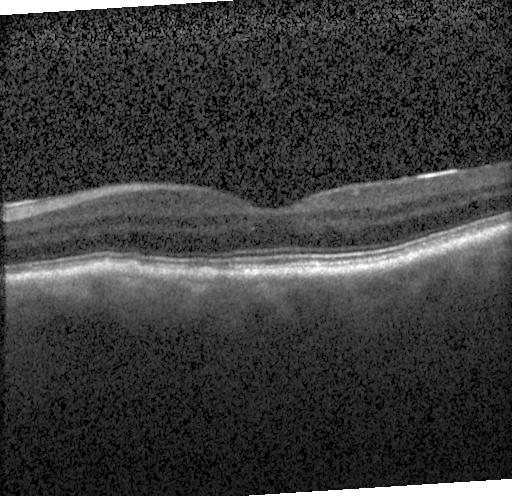 OCT finding: multiple drusen.